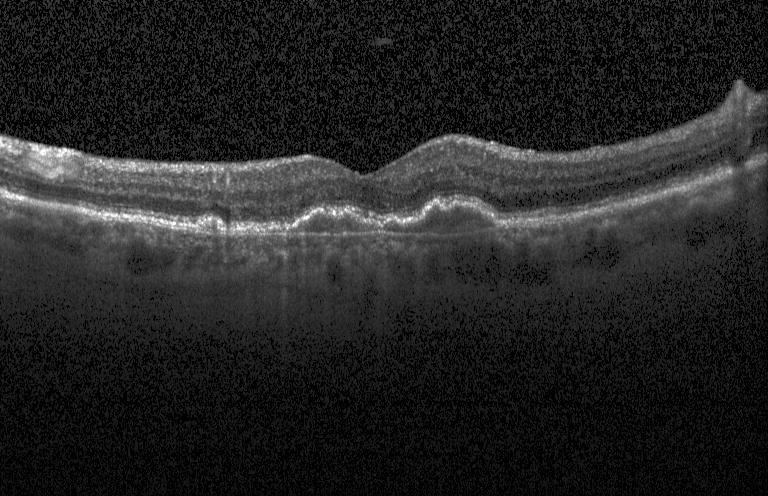
OCT B-scan. Heidelberg Spectralis. Spectral-domain OCT. Fovea-centered — Dx: a choroidal neovascular membrane.